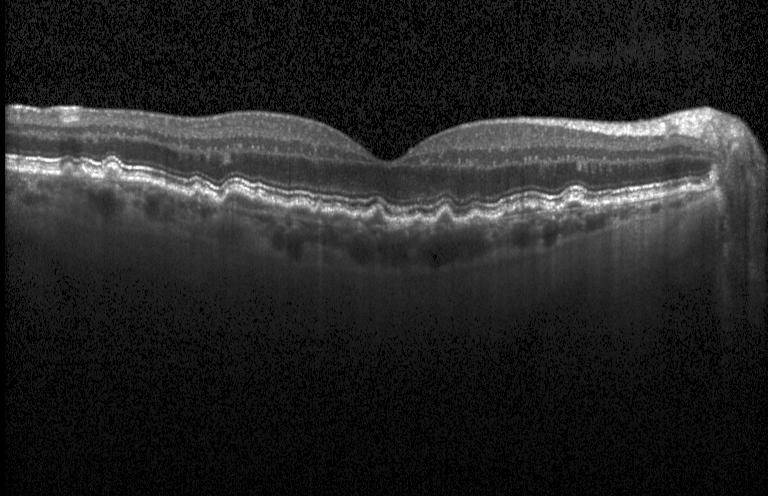
Sub-RPE drusenoid deposits.